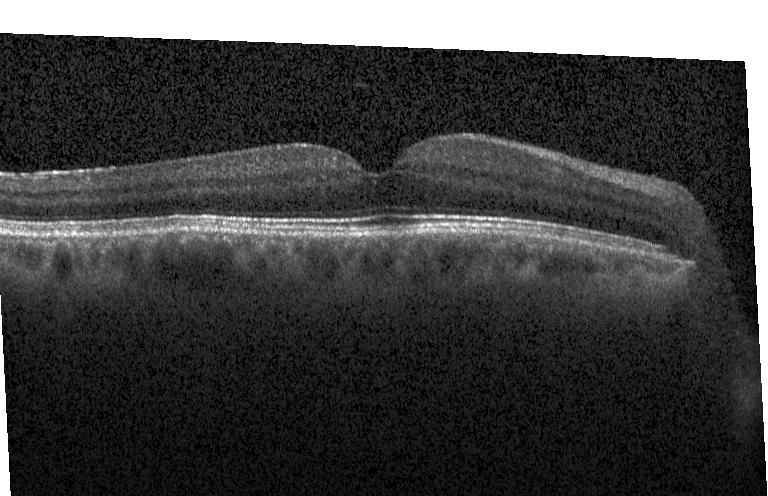 Retinal OCT cross-section; SD-OCT.
Dx: no evidence of choroidal neovascularization, diabetic macular edema, or drusen.